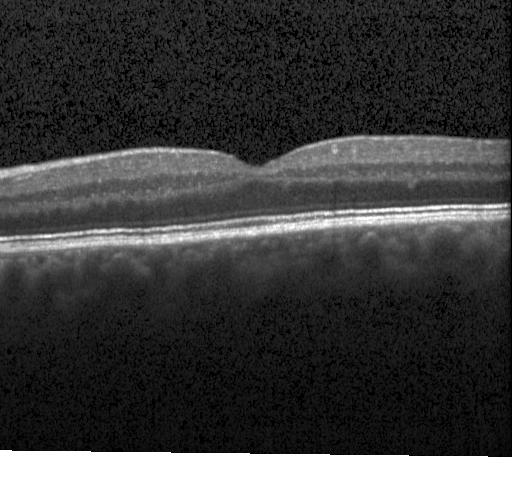

The scan shows no choroidal neovascularization, diabetic macular edema, or drusen.